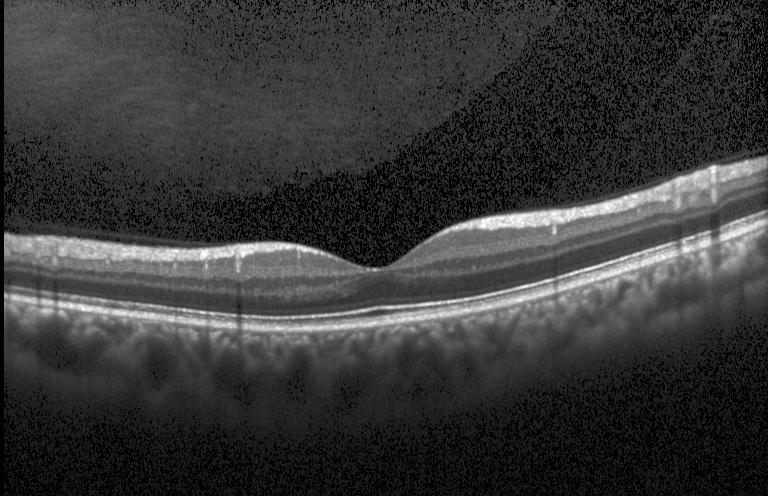
Impression: neither choroidal neovascularization, diabetic macular edema, nor drusen.